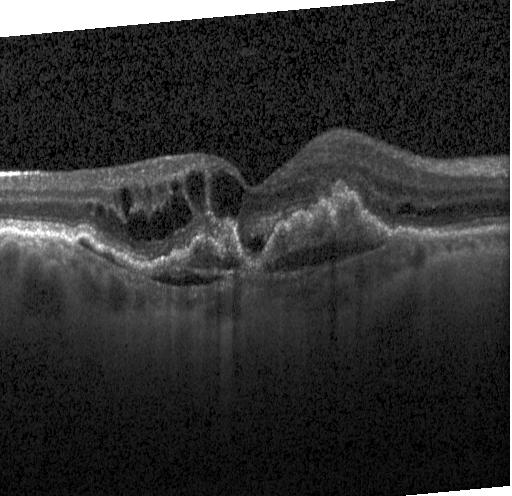 Spectral-domain OCT B-scan: a choroidal neovascular membrane.